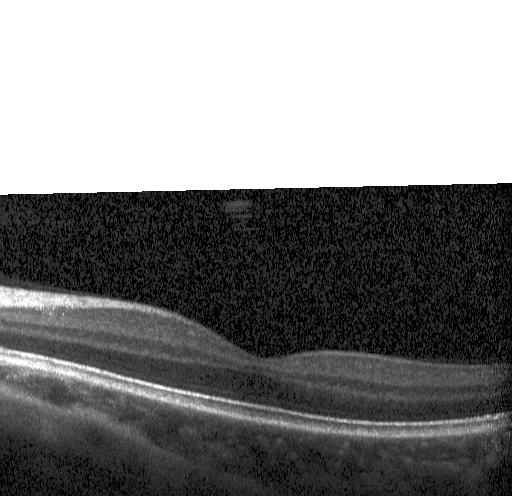 Retinal OCT cross-section.
Diagnosis: no evidence of choroidal neovascularization, diabetic macular edema, or drusen.